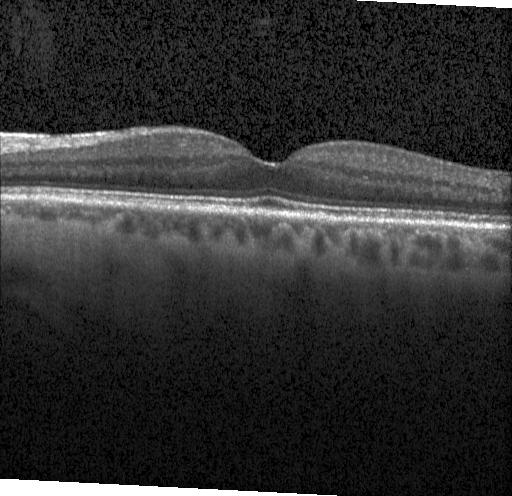 OCT line scan · horizontal scan through the fovea · Heidelberg Spectralis OCT system.
Dx: no choroidal neovascularization, no diabetic macular edema, and no drusen.